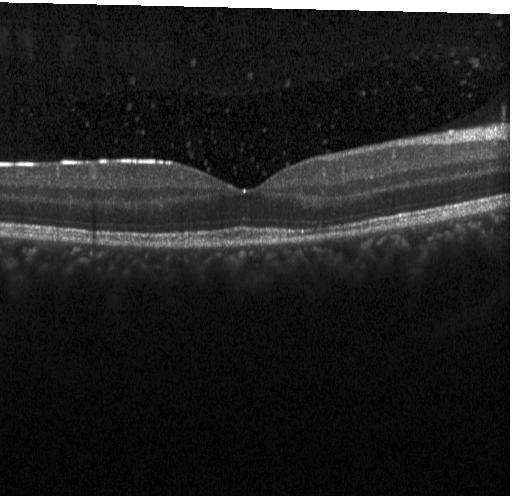 Acquired on a Heidelberg Spectralis; centered on the fovea; optical coherence tomography scan. Diagnosis: no choroidal neovascularization, no diabetic macular edema, and no drusen.